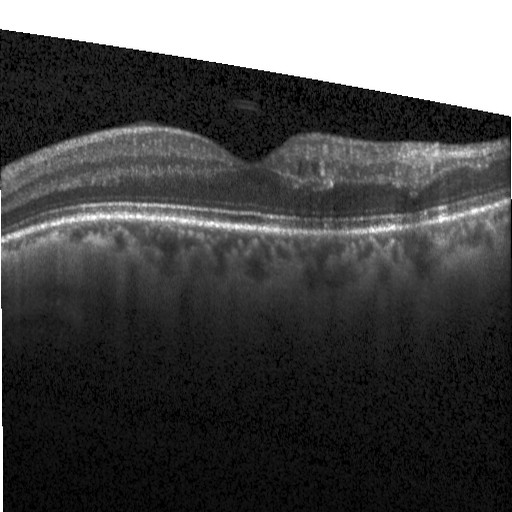 Spectral-domain OCT; through the macula; Heidelberg Spectralis; optical coherence tomography scan. OCT finding: diabetic macular edema.